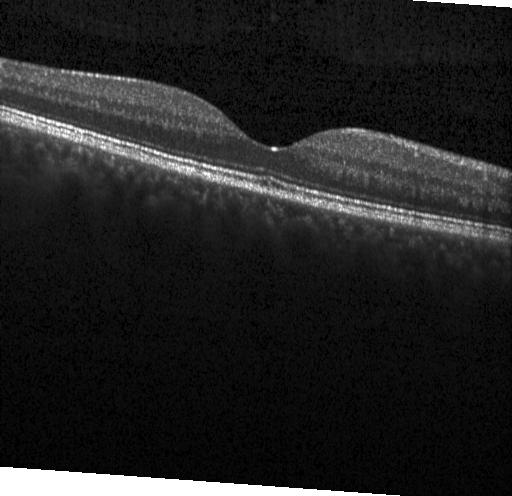
OCT B-scan, SD-OCT, instrument: Heidelberg Spectralis. Finding: no evidence of choroidal neovascularization, diabetic macular edema, or drusen.